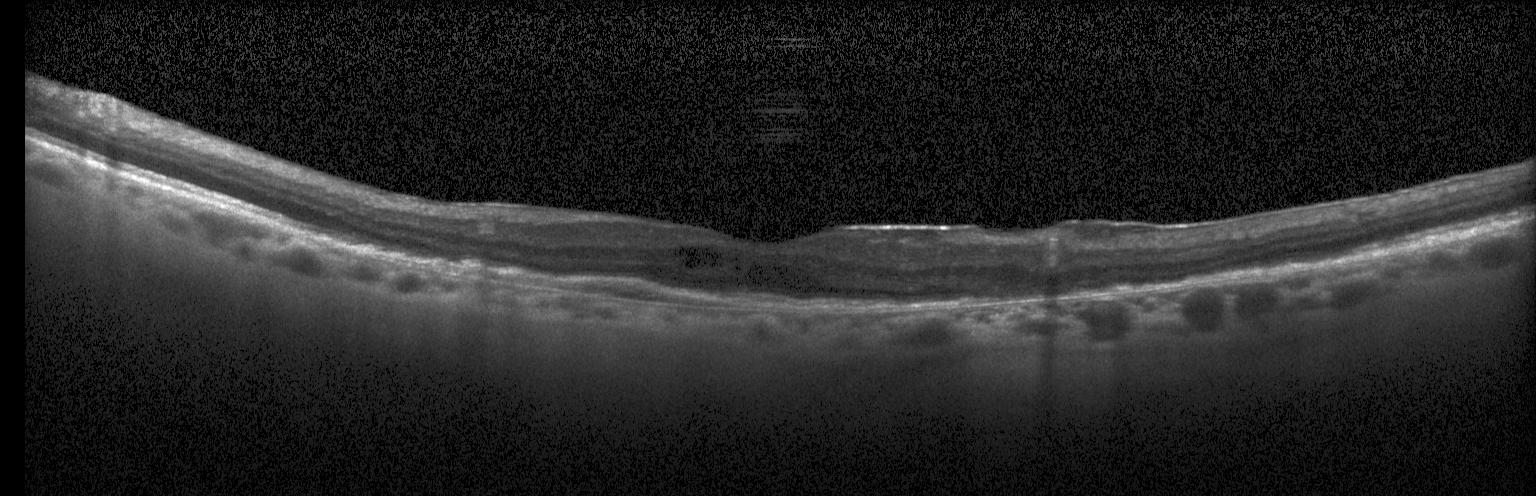
SD-OCT, Heidelberg Spectralis OCT system, OCT line scan.
Impression: choroidal neovascularization (CNV).